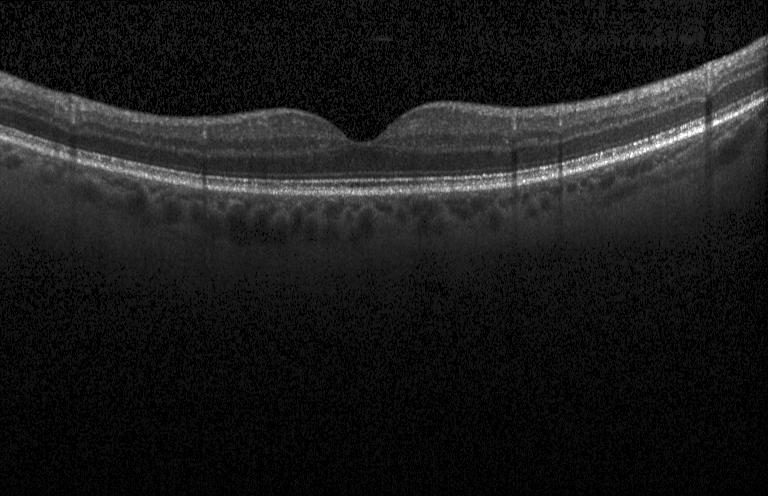

Acquired on a Heidelberg Spectralis · OCT line scan — This B-scan demonstrates neither CNV, DME, nor drusen.